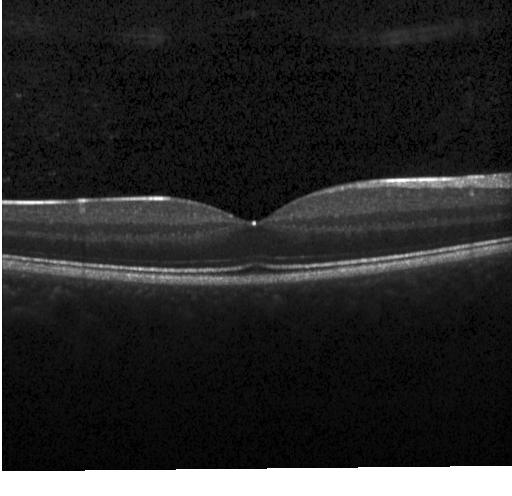
Finding: neither choroidal neovascularization, diabetic macular edema, nor drusen.